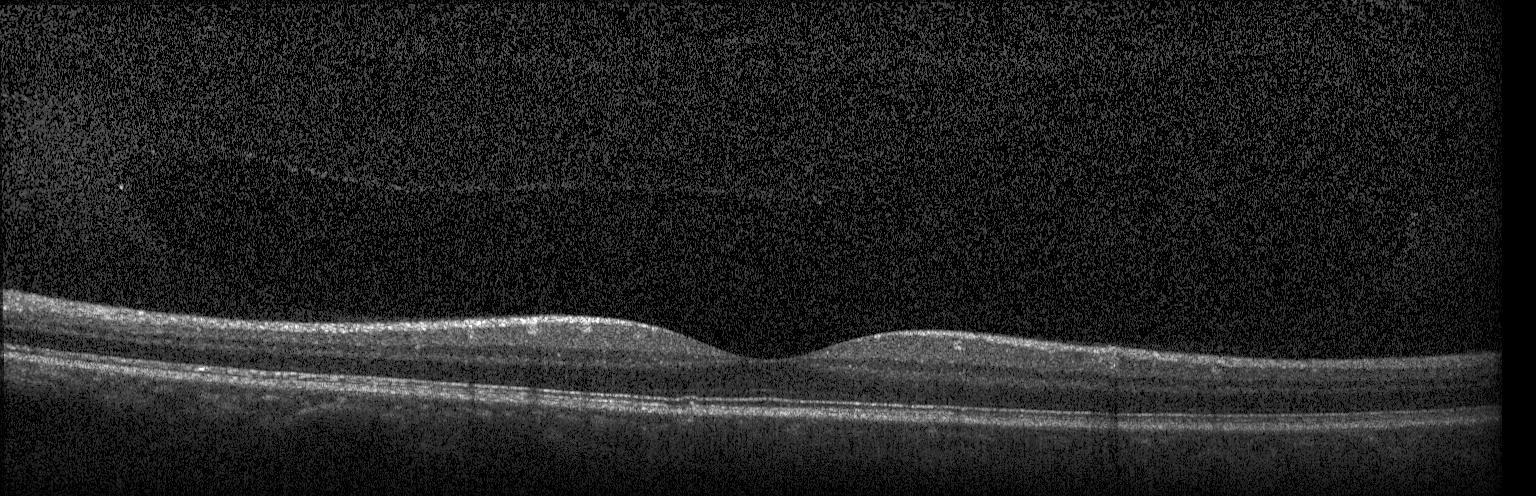
Acquired on a Heidelberg Spectralis; optical coherence tomography B-scan; horizontal scan through the fovea; spectral-domain OCT — Finding: no choroidal neovascularization, diabetic macular edema, or drusen.